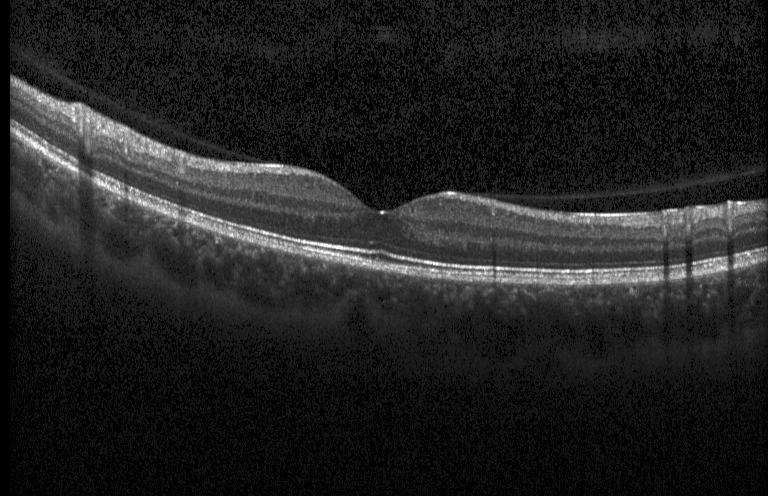
Macular OCT: no choroidal neovascularization, no diabetic macular edema, and no drusen.